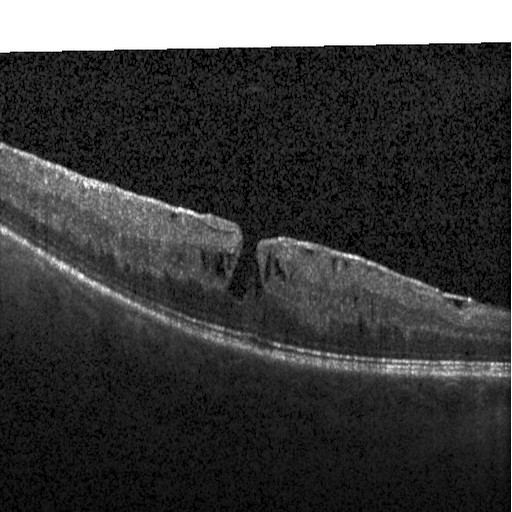

SD-OCT, optical coherence tomography scan, instrument: Heidelberg Spectralis — Impression: diabetic macular edema (DME).